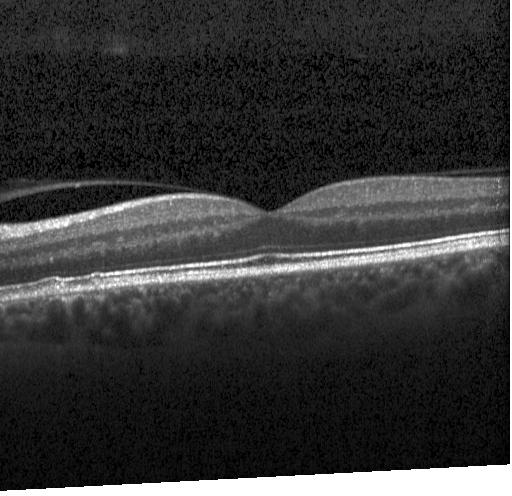
Spectral-domain OCT; OCT line scan; acquired on a Heidelberg Spectralis — Impression: no choroidal neovascularization, diabetic macular edema, or drusen.